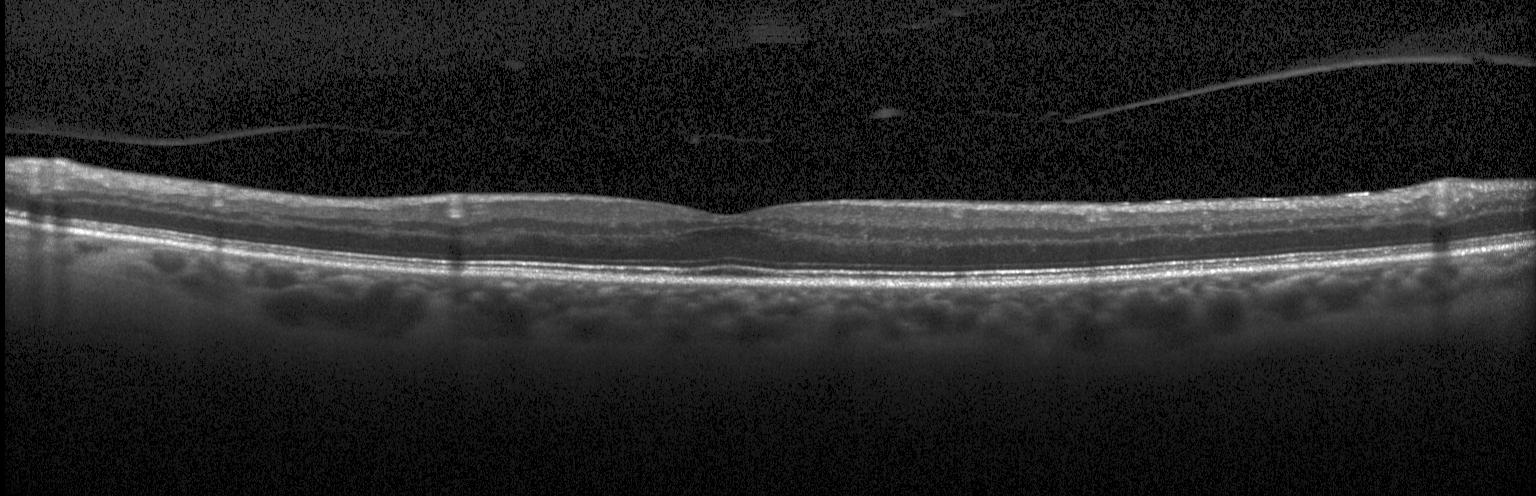 OCT B-scan, fovea-centered, Heidelberg Spectralis, spectral-domain optical coherence tomography.
Diagnosis: neither choroidal neovascularization, diabetic macular edema, nor drusen.